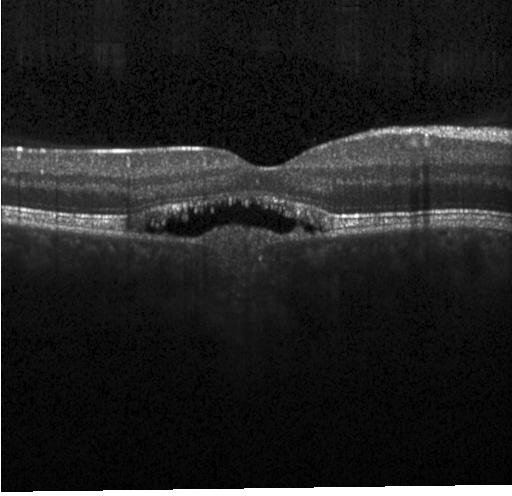 OCT scan showing a choroidal neovascular membrane.